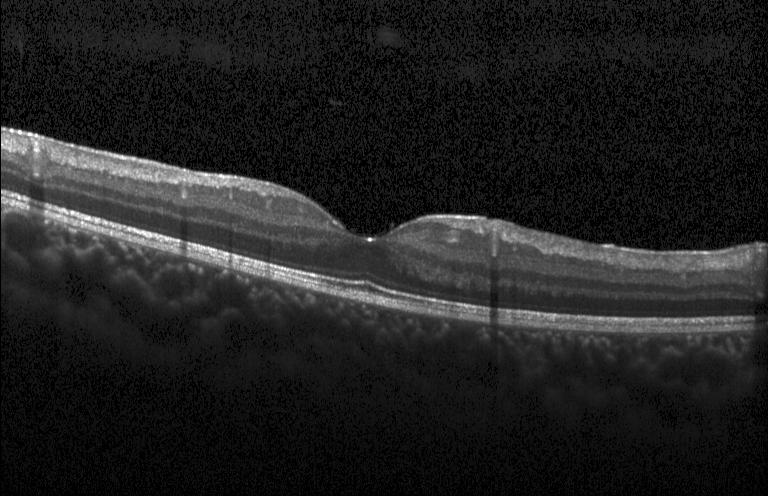

Retinal OCT B-scan, spectral-domain optical coherence tomography.
The scan shows no choroidal neovascularization, diabetic macular edema, or drusen.